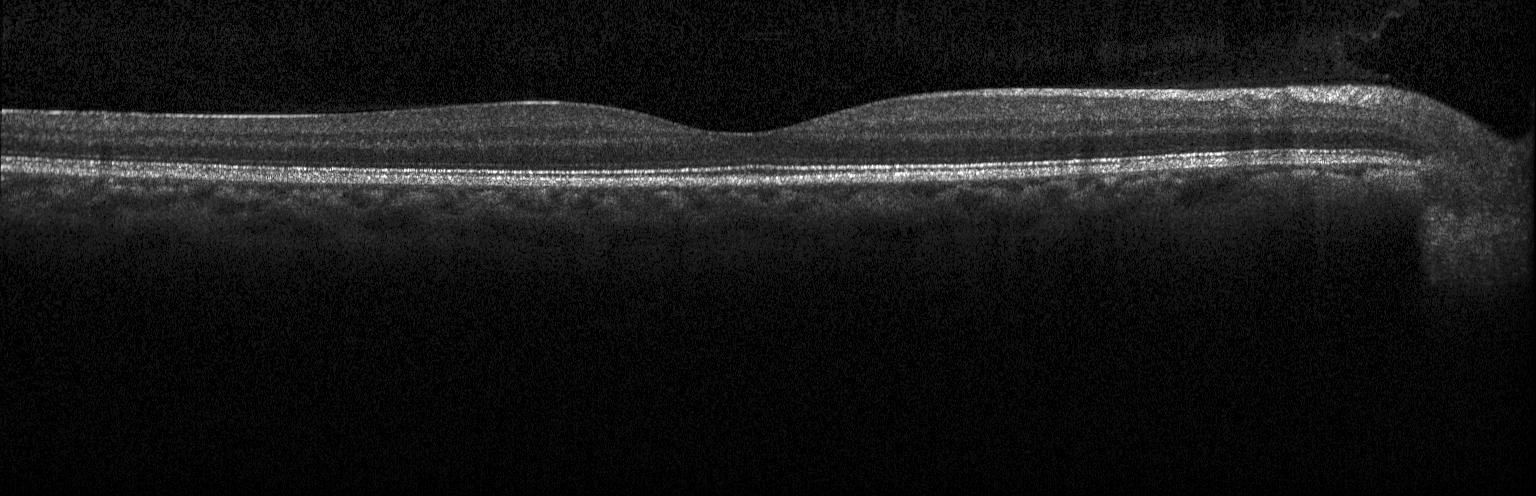 SD-OCT; optical coherence tomography scan. Assessment: neither choroidal neovascularization, diabetic macular edema, nor drusen.